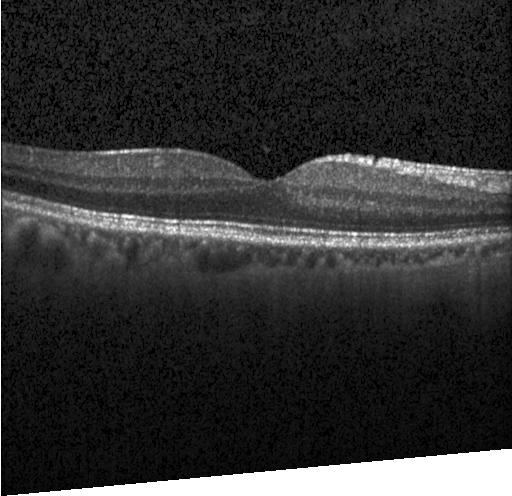
Retinal OCT cross-section · spectral-domain OCT. This B-scan demonstrates no evidence of CNV, DME, or drusen.